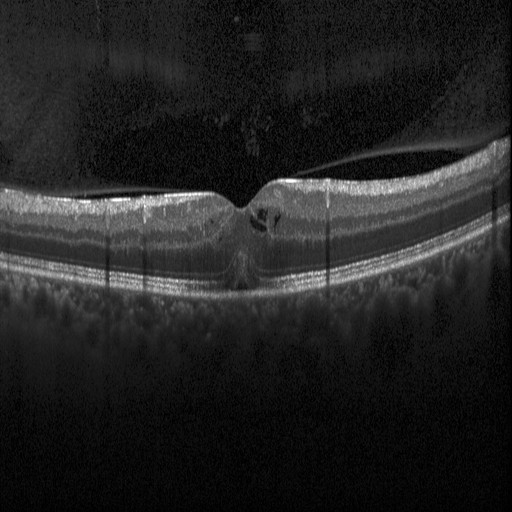

Heidelberg Spectralis OCT system. Fovea-centered. OCT line scan
OCT finding: diabetic macular edema (DME).